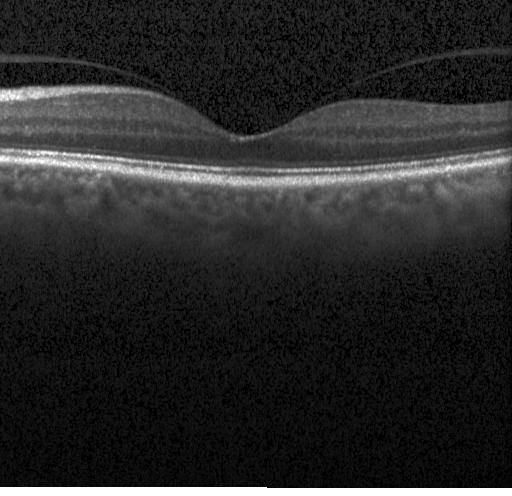

Optical coherence tomography B-scan; macular scan; Heidelberg Spectralis; spectral-domain optical coherence tomography.
Assessment: no choroidal neovascularization, diabetic macular edema, or drusen.